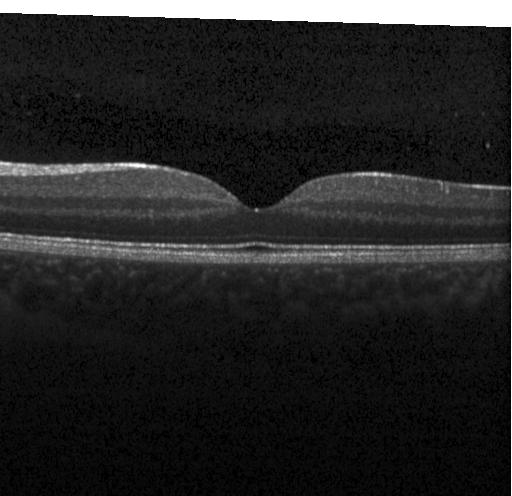
Dx: no evidence of CNV, DME, or drusen.